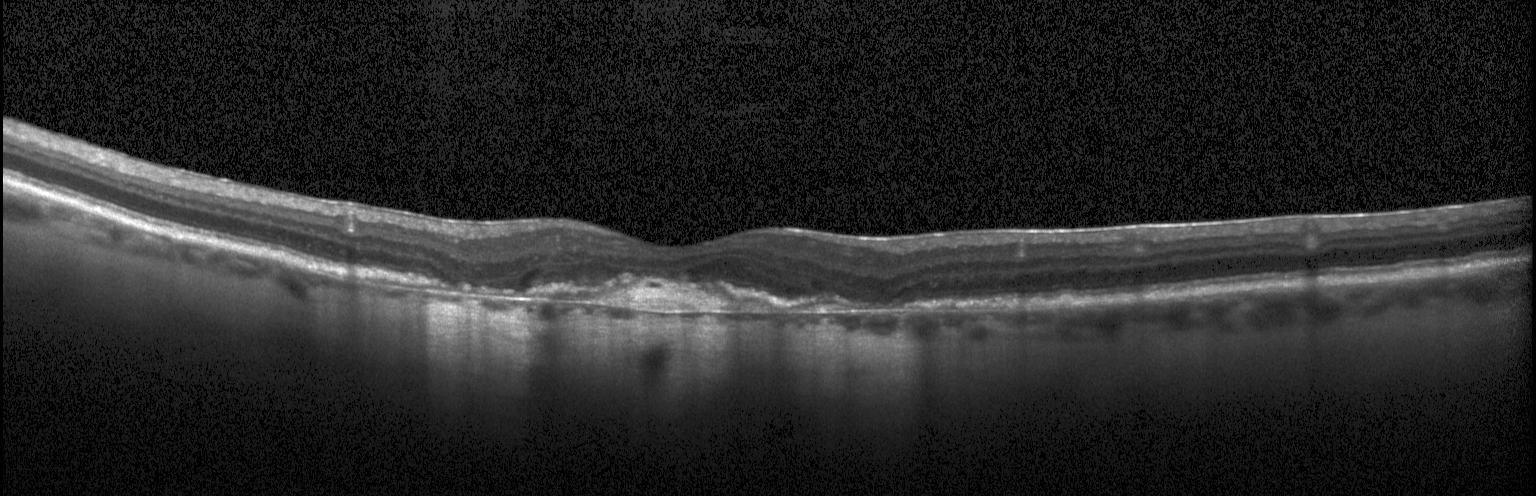 Retinal OCT cross-section — Diagnosis: CNV.